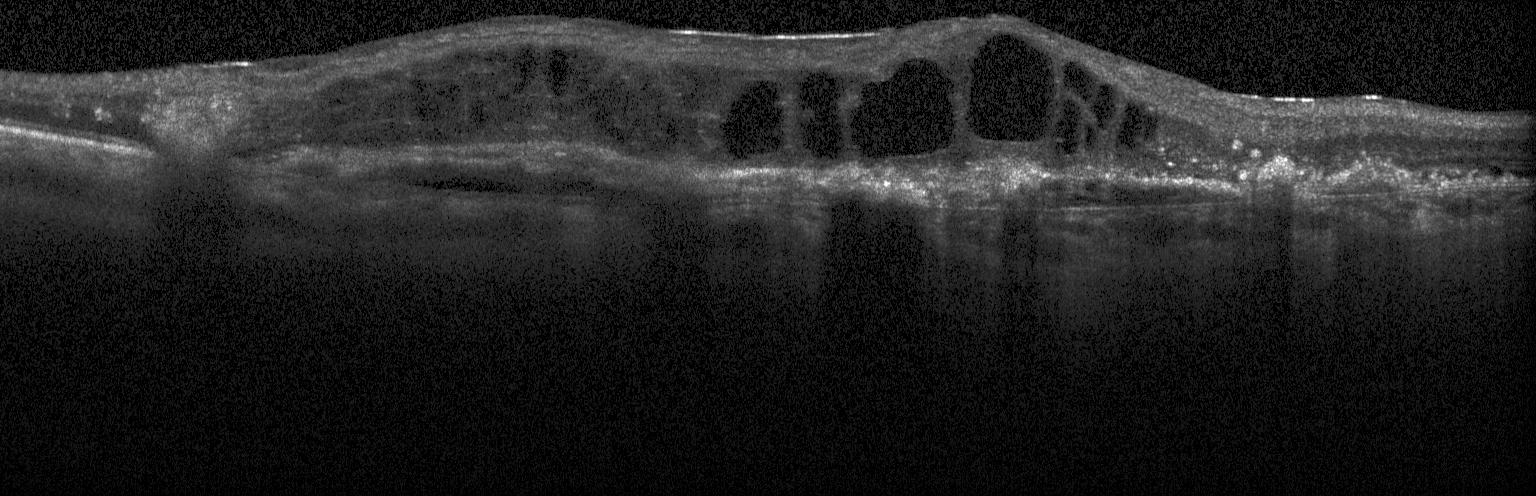 This B-scan demonstrates CNV.